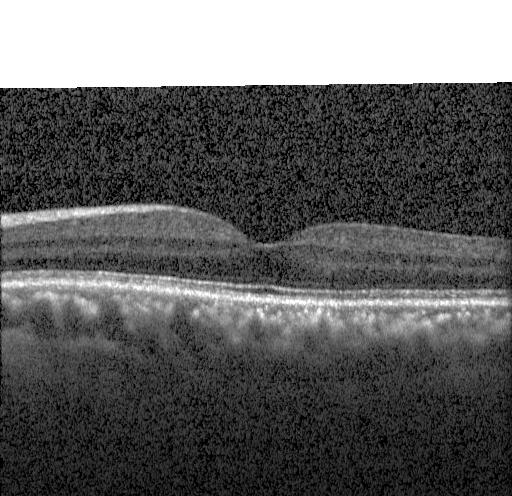
OCT B-scan. Finding: no choroidal neovascularization, diabetic macular edema, or drusen.